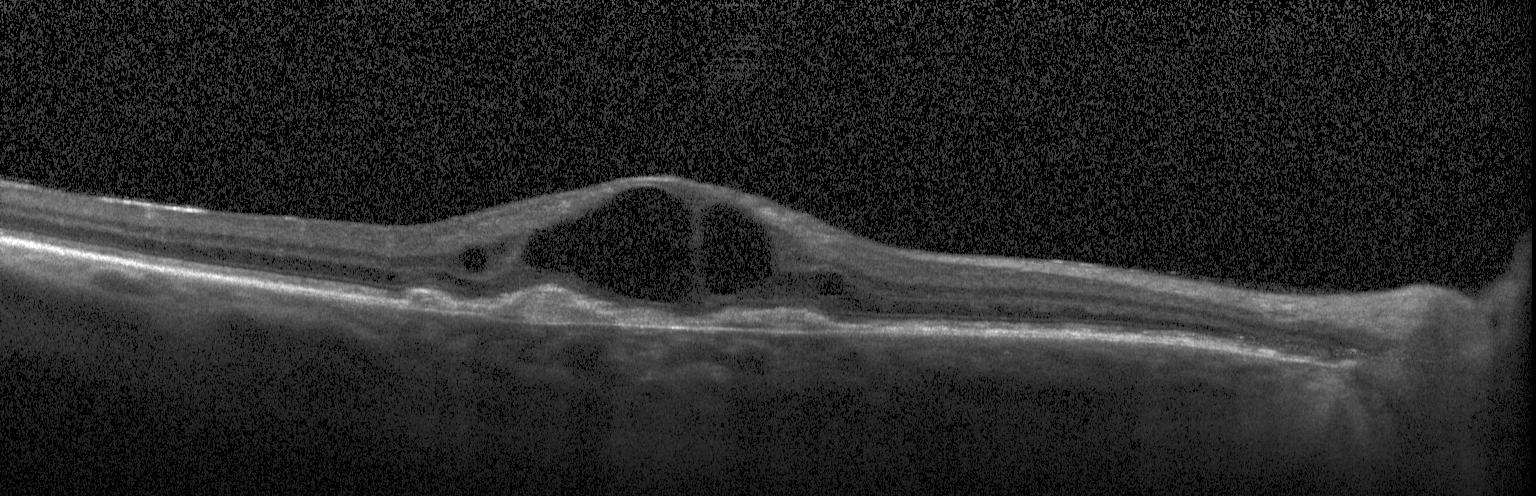

Retinal OCT B-scan, macular scan, instrument: Heidelberg Spectralis — OCT finding: a choroidal neovascular membrane.